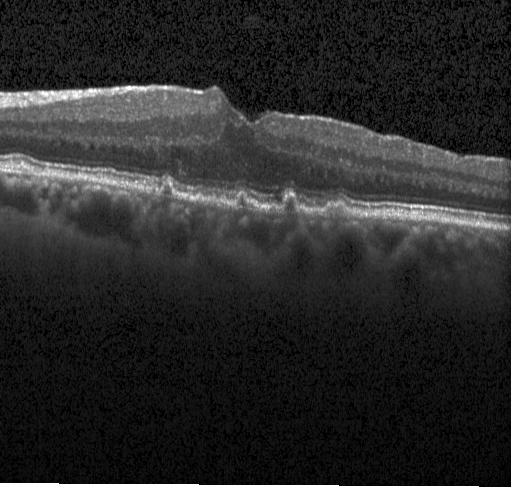

OCT B-scan showing sub-RPE drusenoid deposits.